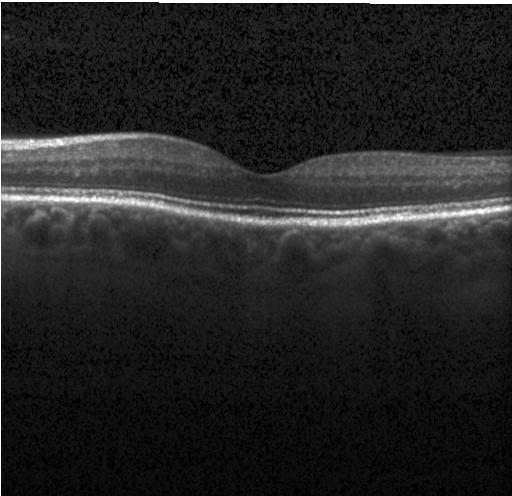
Macular scan. Spectral-domain OCT. OCT line scan. Acquired on a Heidelberg Spectralis
OCT finding: neither choroidal neovascularization, diabetic macular edema, nor drusen.